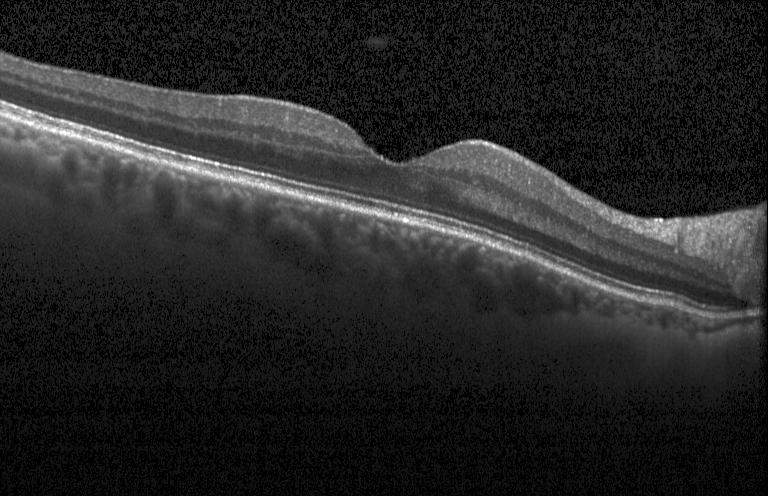
Retinal OCT B-scan, spectral-domain optical coherence tomography
Diagnosis: no evidence of choroidal neovascularization, diabetic macular edema, or drusen.